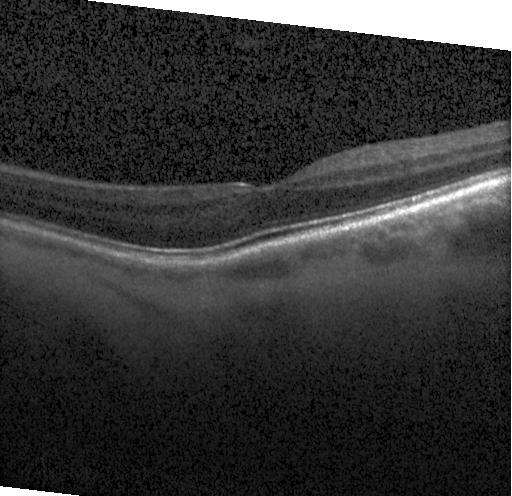

Diagnosis: no choroidal neovascularization, diabetic macular edema, or drusen.